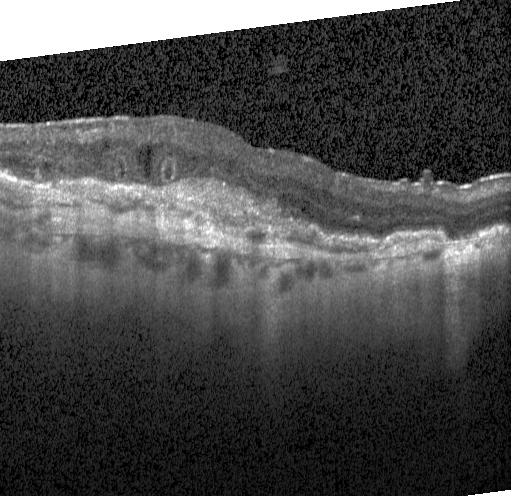

Centered on the fovea, spectral-domain OCT, optical coherence tomography scan — Diagnosis: a choroidal neovascular membrane.